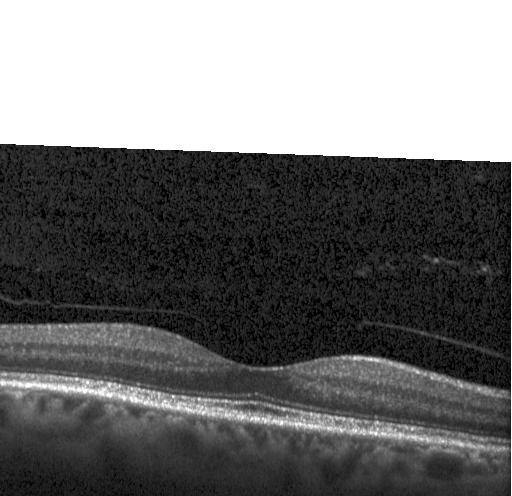

Spectral-domain OCT · through the macula · Heidelberg Spectralis · OCT B-scan. OCT finding: no choroidal neovascularization, no diabetic macular edema, and no drusen.